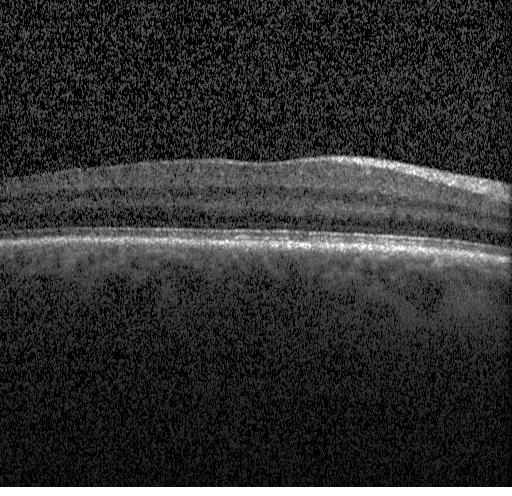

SD-OCT. Through the macula. Retinal OCT cross-section
No choroidal neovascularization, no diabetic macular edema, and no drusen.